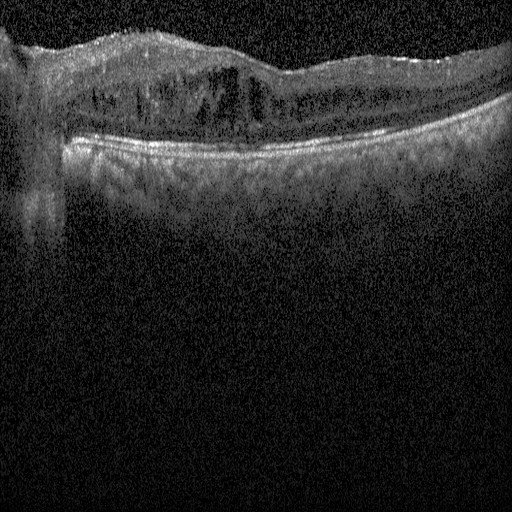
Spectral-domain OCT, optical coherence tomography scan — Diagnosis: diabetic macular edema.